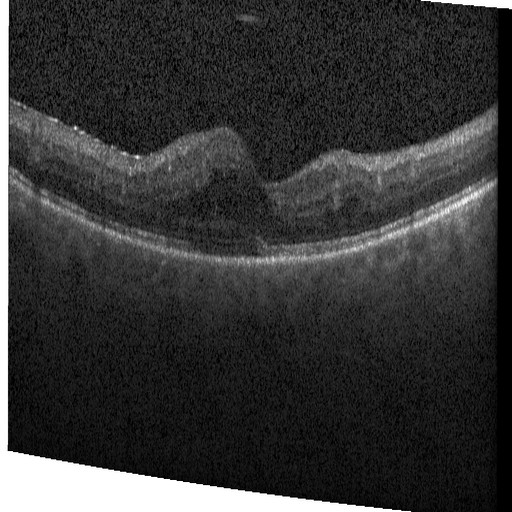

Spectral-domain OCT · through the macula · OCT line scan.
Diabetic macular edema (DME).